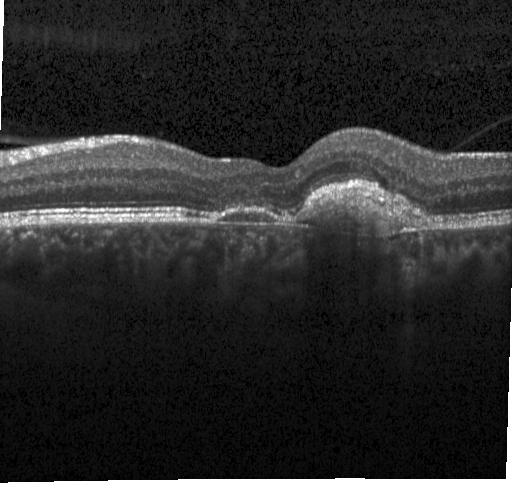
Optical coherence tomography scan — Impression: a choroidal neovascular membrane.